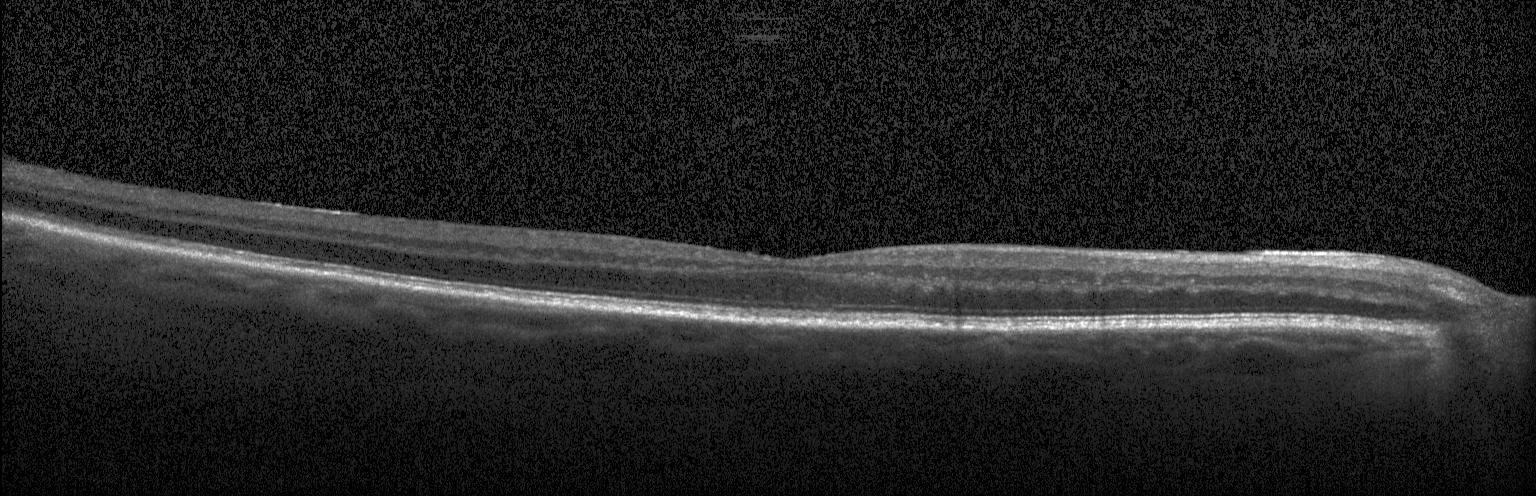 Optical coherence tomography scan. Heidelberg Spectralis — The scan shows no choroidal neovascularization, no diabetic macular edema, and no drusen.